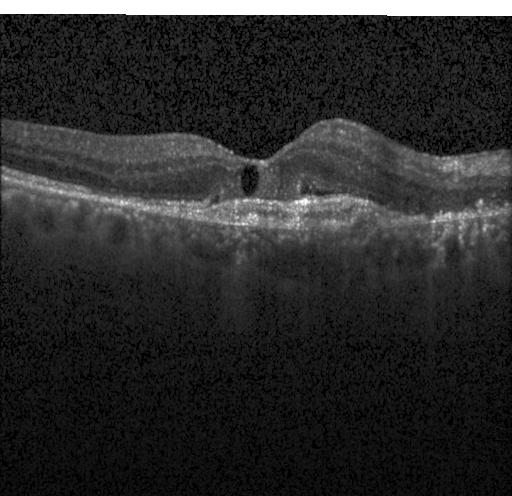
Macular OCT demonstrating choroidal neovascularization (CNV).